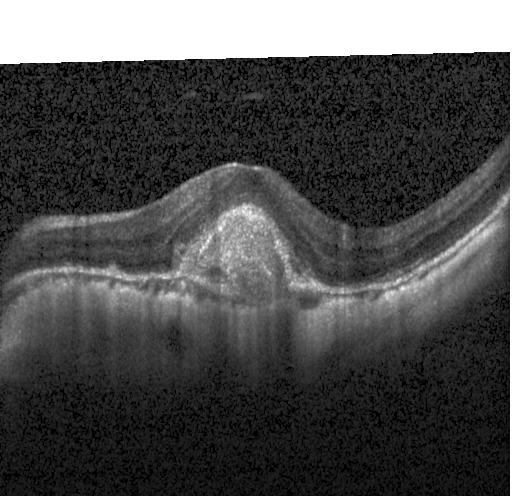

OCT B-scan
Diagnosis: choroidal neovascularization.